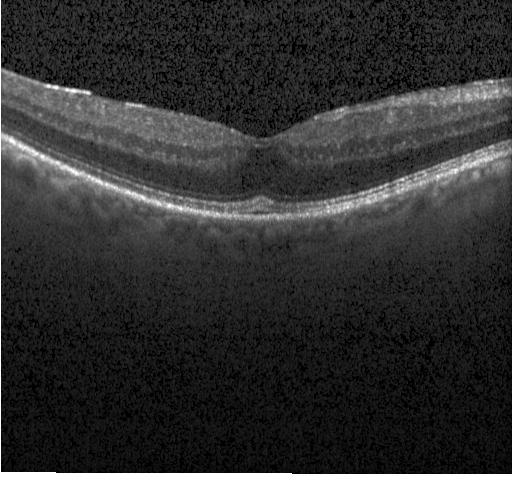 No choroidal neovascularization, no diabetic macular edema, and no drusen.